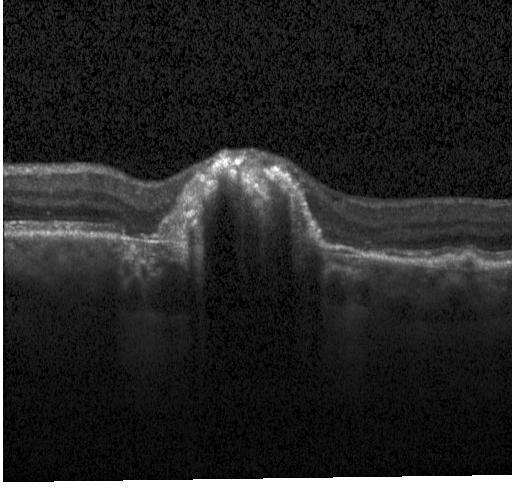 OCT finding: a choroidal neovascular membrane.